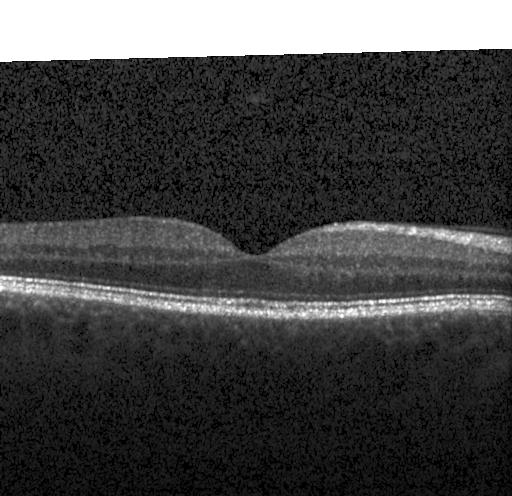
Instrument: Heidelberg Spectralis, SD-OCT, optical coherence tomography scan.
This B-scan demonstrates neither choroidal neovascularization, diabetic macular edema, nor drusen.